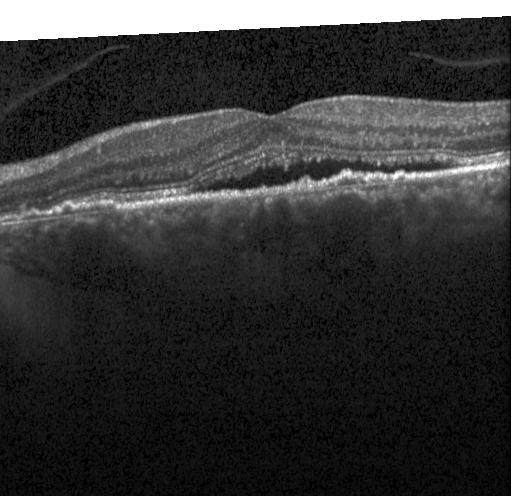

Finding: choroidal neovascularization.